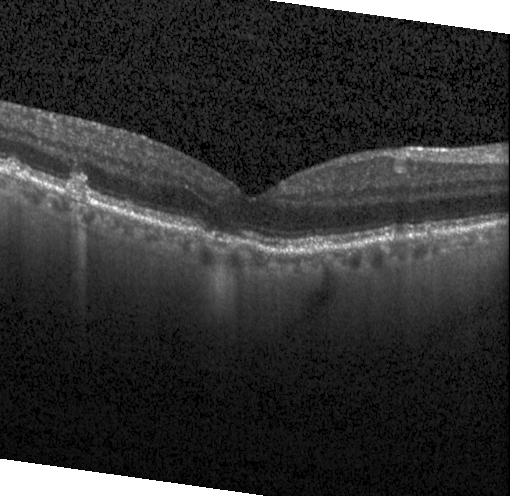

Through the macula, optical coherence tomography B-scan, acquired on a Heidelberg Spectralis, spectral-domain OCT. Diagnosis: drusen.